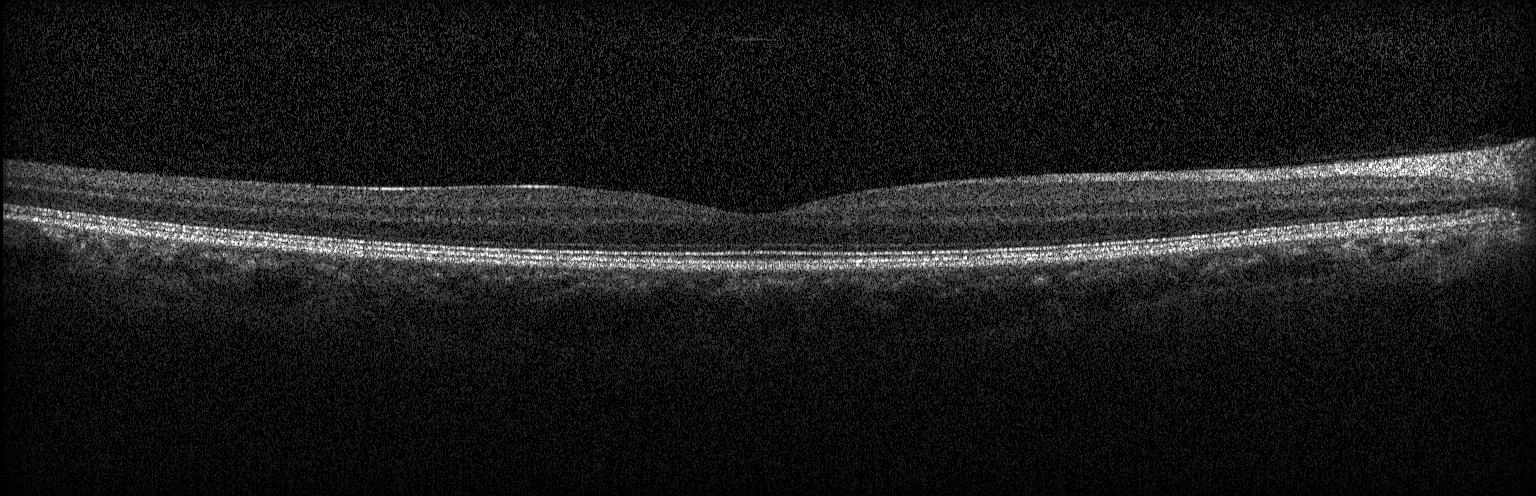 Dx: no evidence of choroidal neovascularization, diabetic macular edema, or drusen.